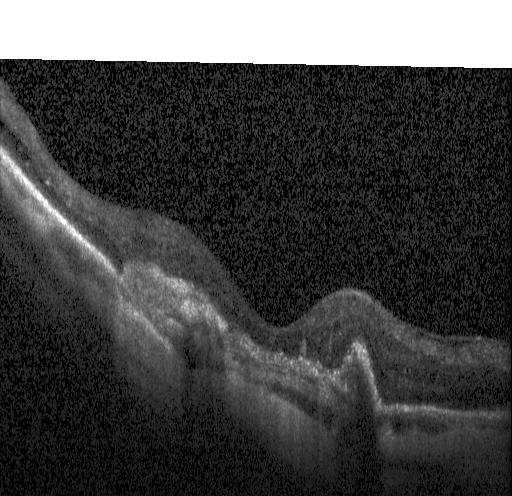 Retinal OCT B-scan; spectral-domain OCT.
This B-scan demonstrates a choroidal neovascular membrane.